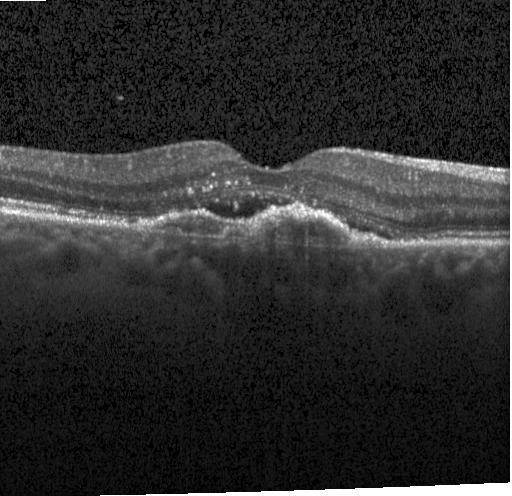
Finding: a choroidal neovascular membrane.